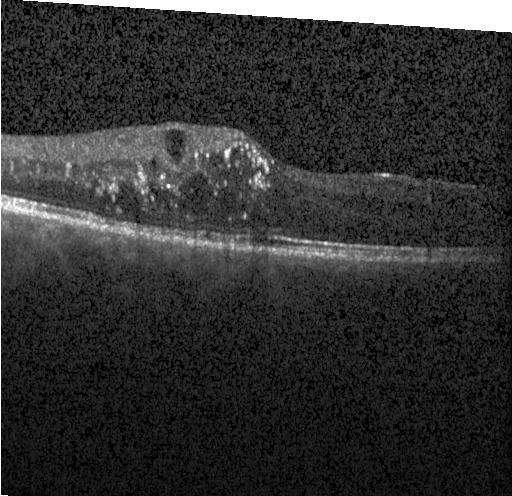
Impression: DME.